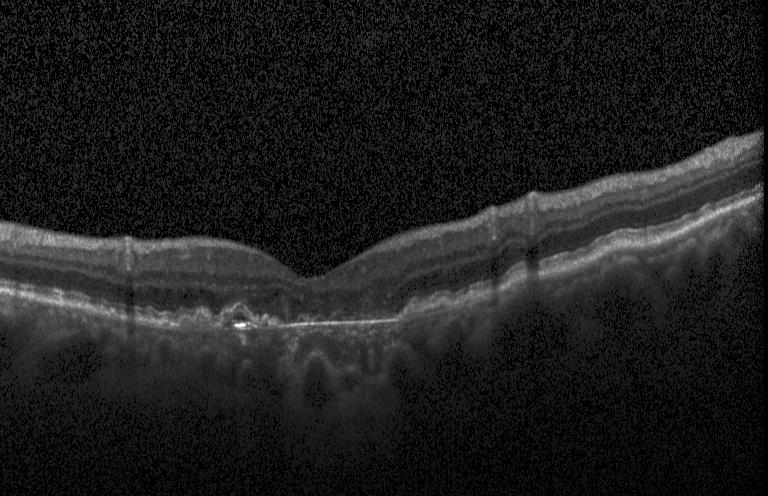

SD-OCT. OCT B-scan
This B-scan demonstrates a choroidal neovascular membrane.